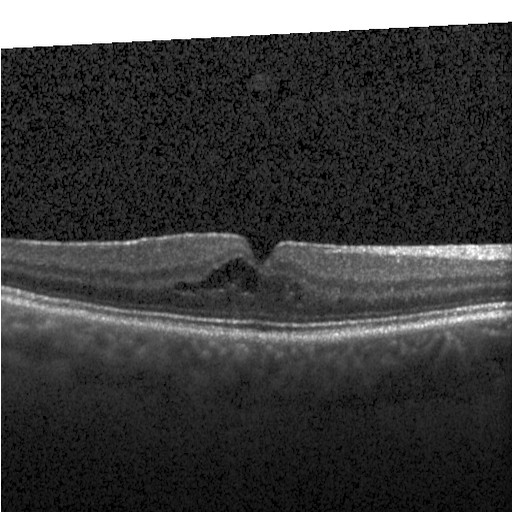
Retinal OCT B-scan, Heidelberg Spectralis, horizontal scan through the fovea, spectral-domain OCT. This B-scan demonstrates diabetic macular edema (DME).